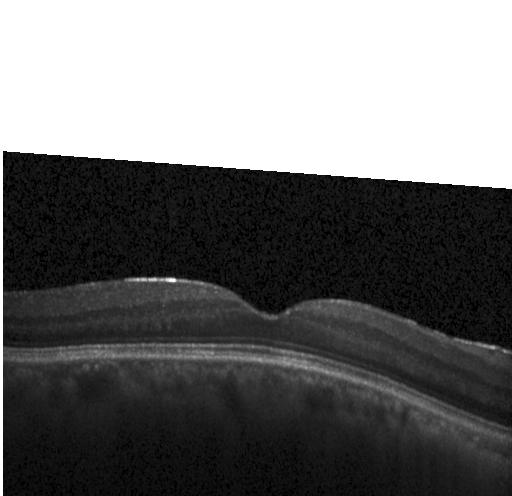

Heidelberg Spectralis; optical coherence tomography scan. Impression: no evidence of CNV, DME, or drusen.